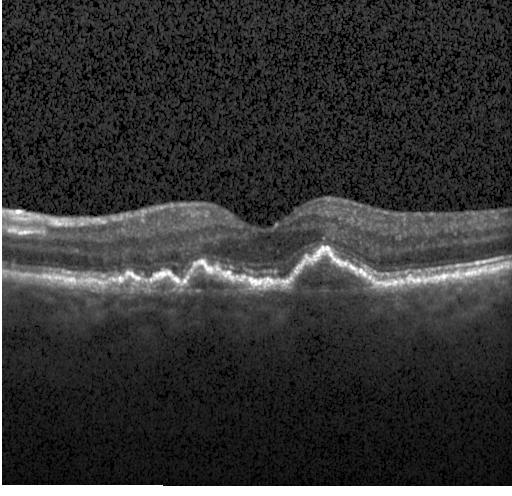

Spectral-domain optical coherence tomography; OCT line scan.
This B-scan demonstrates a choroidal neovascular membrane.